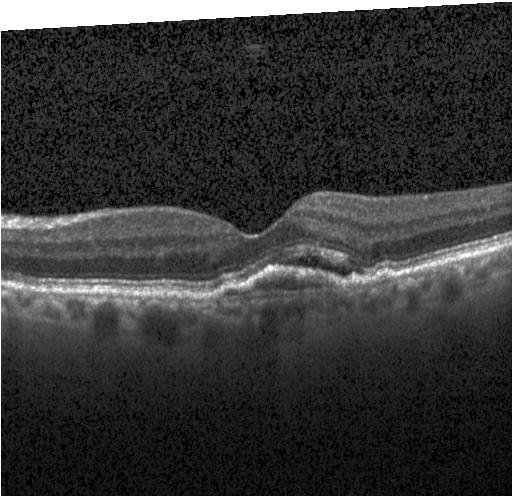
Heidelberg Spectralis OCT system, optical coherence tomography scan, spectral-domain optical coherence tomography
The scan shows choroidal neovascularization (CNV).